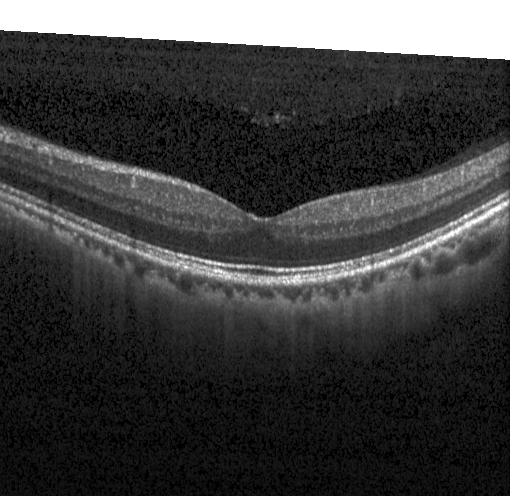 Acquired on a Heidelberg Spectralis; OCT B-scan
Diagnosis: neither choroidal neovascularization, diabetic macular edema, nor drusen.